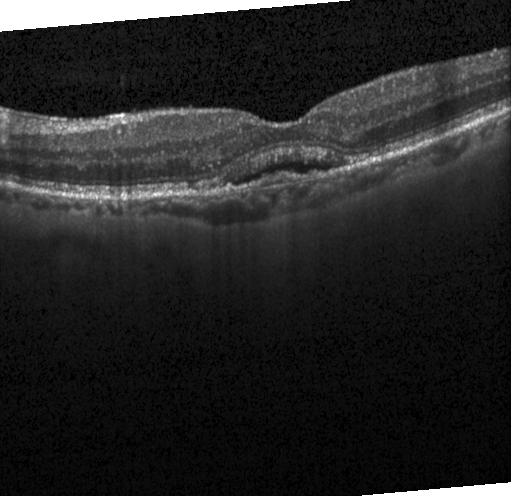
Spectral-domain optical coherence tomography; optical coherence tomography B-scan — Finding: a choroidal neovascular membrane.